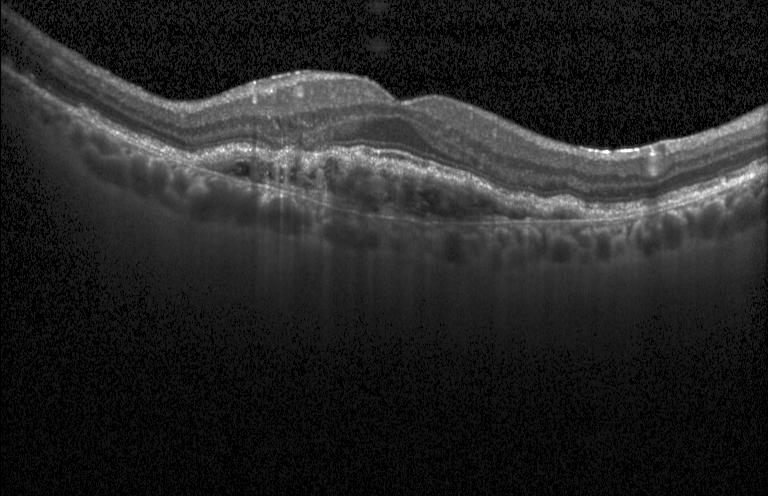 OCT line scan. Choroidal neovascularization.